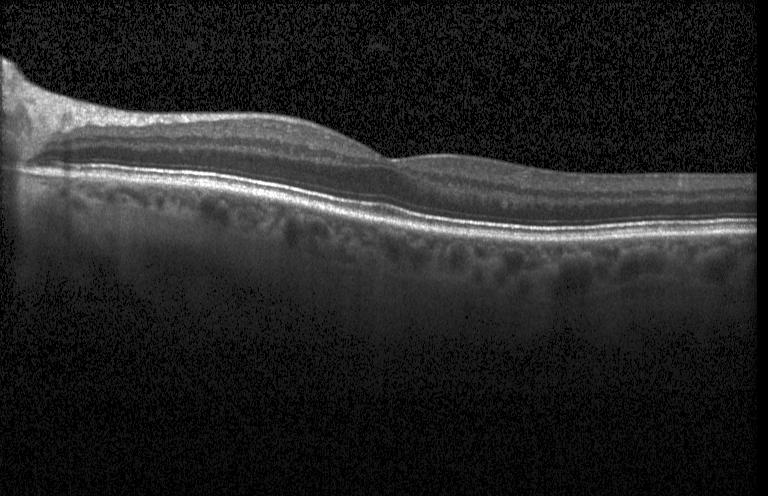 SD-OCT, OCT line scan, macular scan, acquired on a Heidelberg Spectralis
Diagnosis: no CNV, no DME, and no drusen.